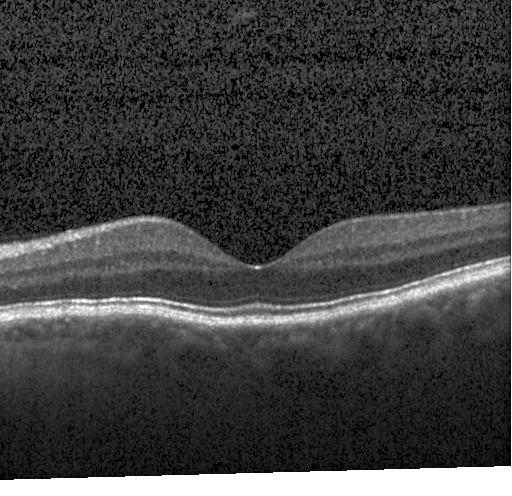 OCT finding: no CNV, no DME, and no drusen.